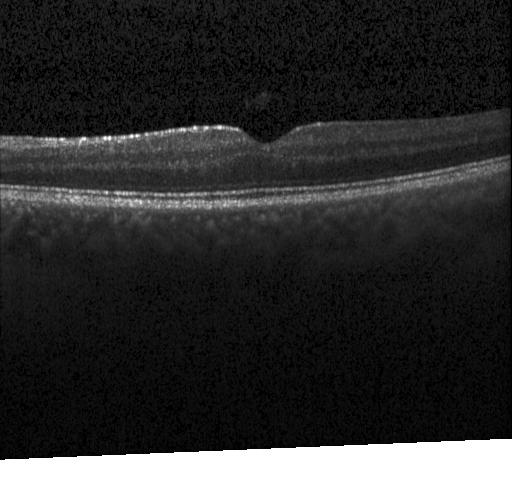

Macular OCT: neither choroidal neovascularization, diabetic macular edema, nor drusen.